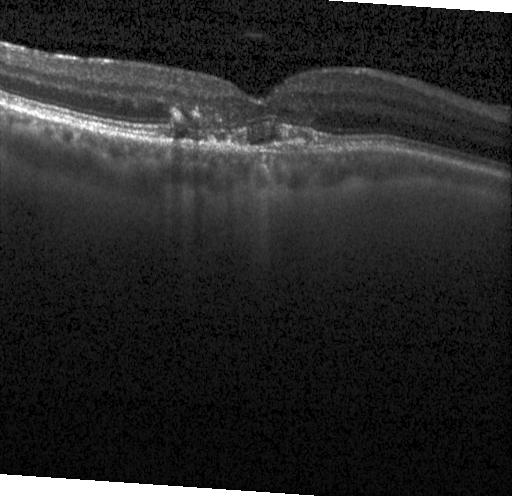 Fovea-centered · retinal OCT cross-section · Heidelberg Spectralis OCT system — Impression: a choroidal neovascular membrane.